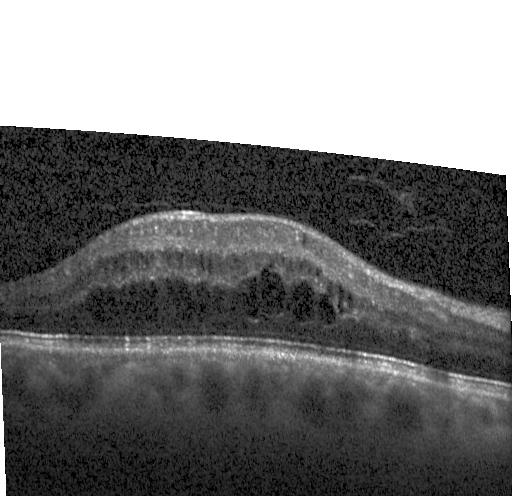

Acquired on a Heidelberg Spectralis; optical coherence tomography scan; spectral-domain OCT; centered on the fovea. Assessment: DME.